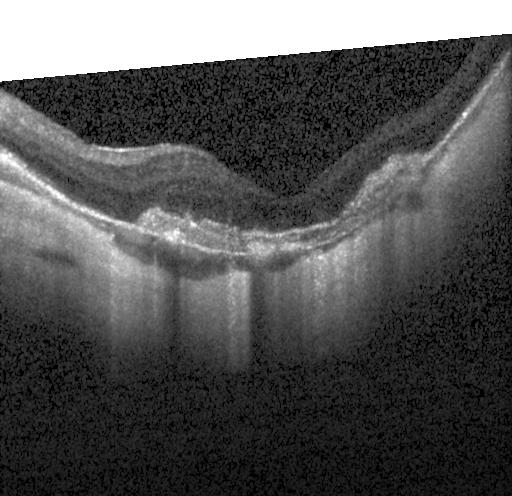 Horizontal scan through the fovea; OCT line scan.
Diagnosis: a choroidal neovascular membrane.